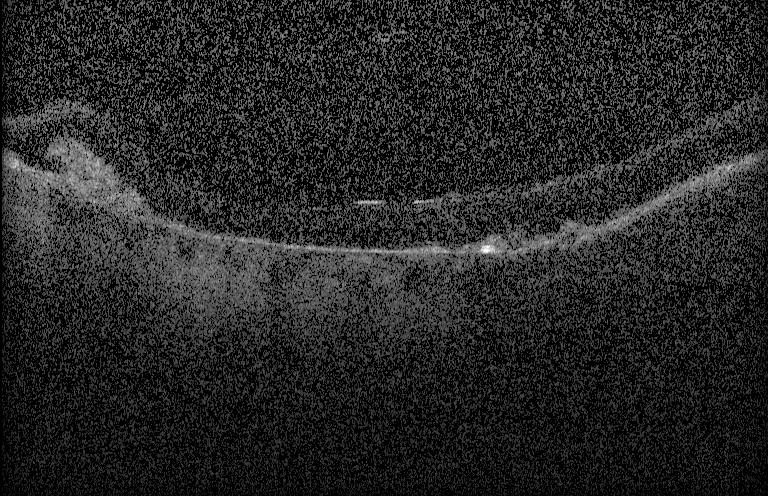

Spectral-domain OCT, optical coherence tomography B-scan
A choroidal neovascular membrane.